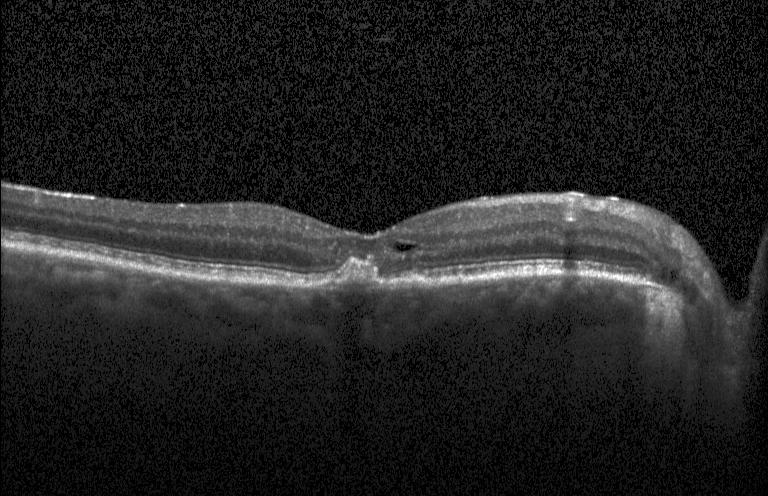

Through the macula · optical coherence tomography scan · SD-OCT.
Assessment: a choroidal neovascular membrane.